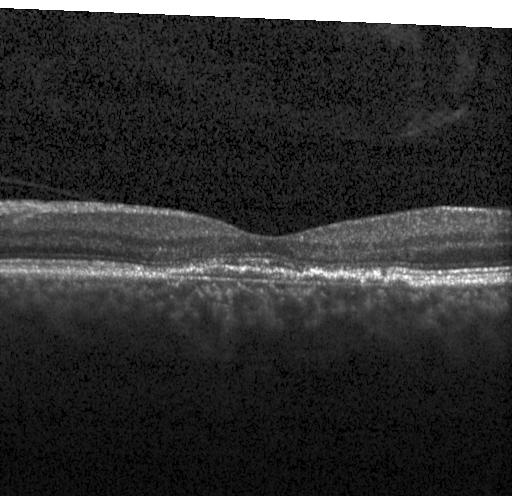 The scan shows a choroidal neovascular membrane.